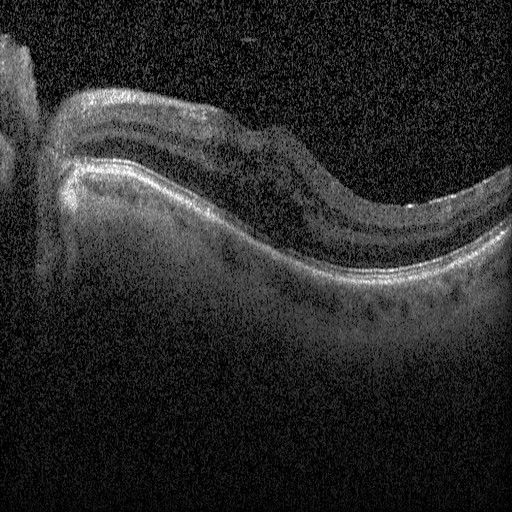

Impression: diabetic macular edema (DME).